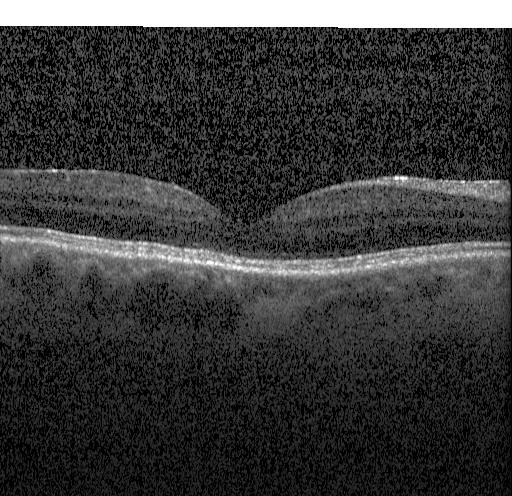 Macular OCT: no CNV, no DME, and no drusen.